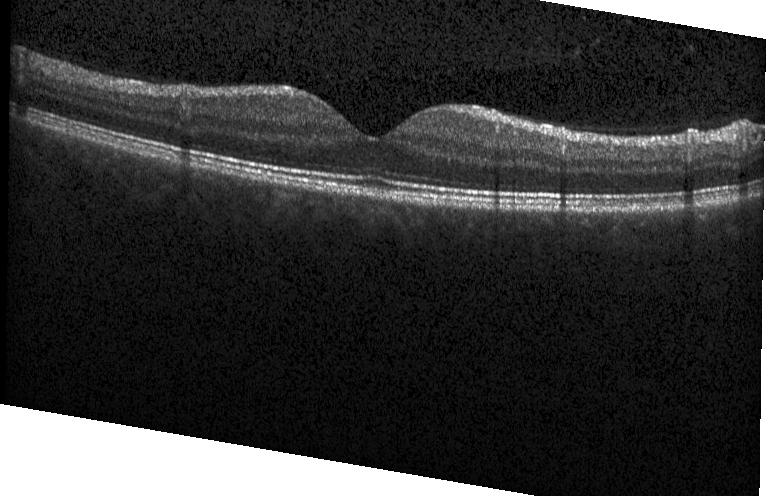 Macular scan, OCT B-scan
Assessment: neither CNV, DME, nor drusen.